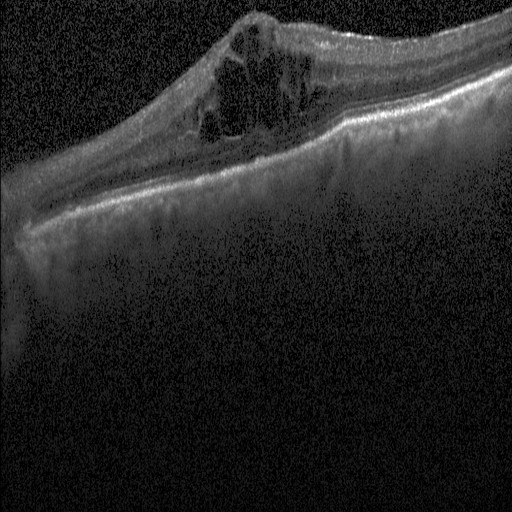

Optical coherence tomography scan, acquired on a Heidelberg Spectralis, centered on the fovea, spectral-domain optical coherence tomography.
Assessment: DME.